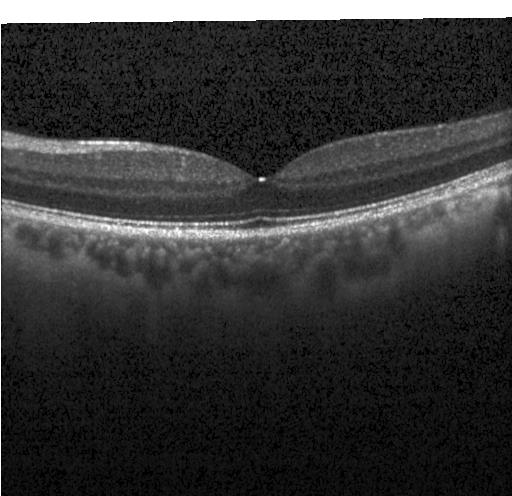
SD-OCT. Acquired on a Heidelberg Spectralis. Optical coherence tomography B-scan.
The scan shows no choroidal neovascularization, diabetic macular edema, or drusen.